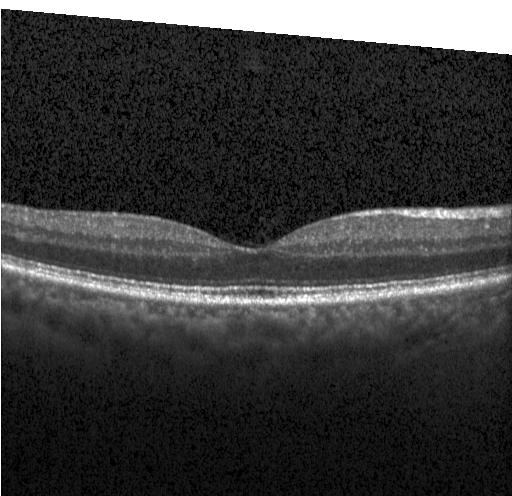 Optical coherence tomography scan · spectral-domain OCT.
Diagnosis: no evidence of choroidal neovascularization, diabetic macular edema, or drusen.